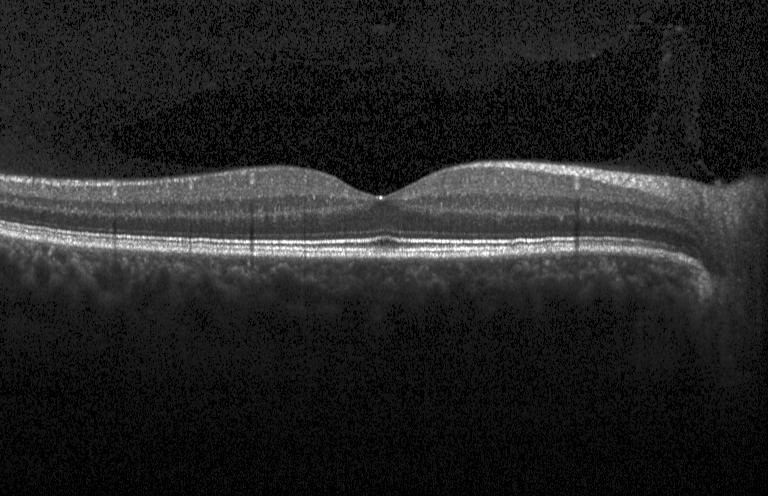

SD-OCT. Optical coherence tomography scan. Through the macula. No evidence of CNV, DME, or drusen.